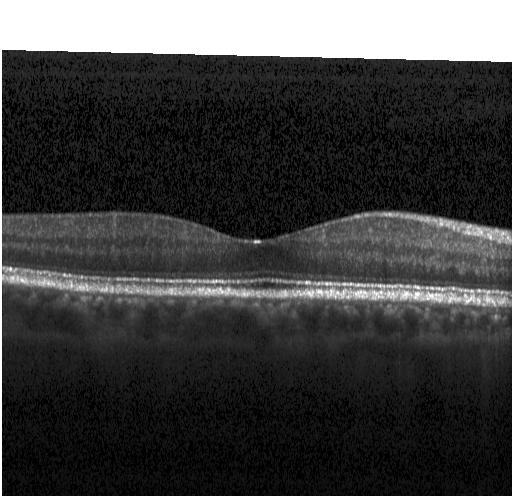 OCT B-scan · macular scan
Dx: neither choroidal neovascularization, diabetic macular edema, nor drusen.